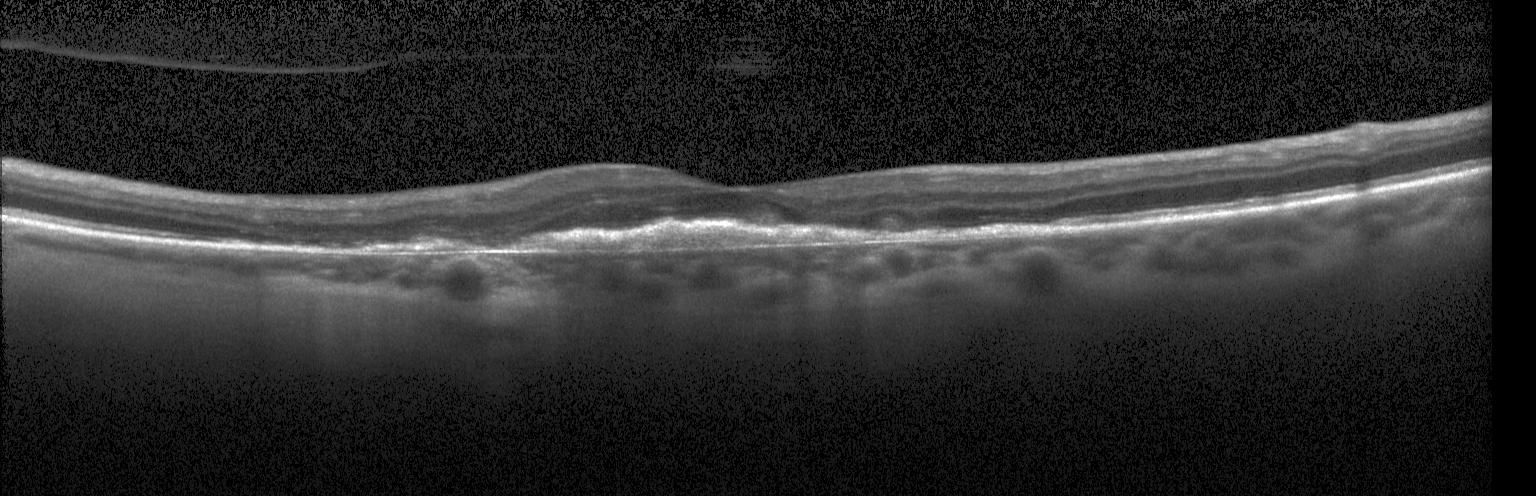 OCT B-scan; acquired on a Heidelberg Spectralis.
OCT finding: a choroidal neovascular membrane.